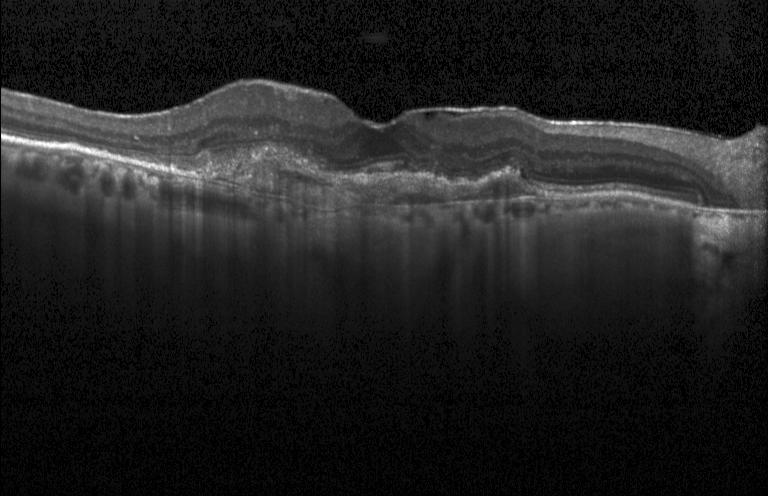

Dx: a choroidal neovascular membrane.